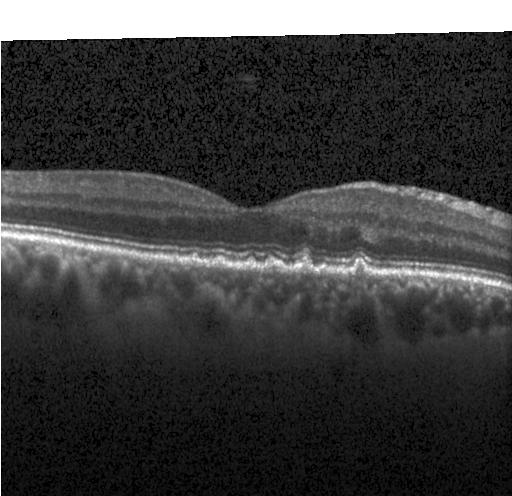

Impression: sub-RPE drusenoid deposits.